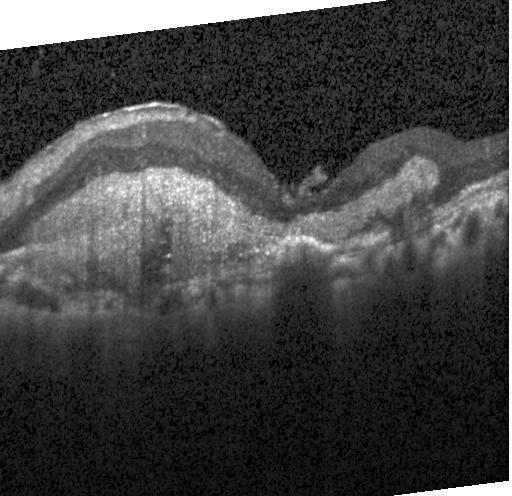

Retinal OCT cross-section; SD-OCT. This B-scan demonstrates choroidal neovascularization.